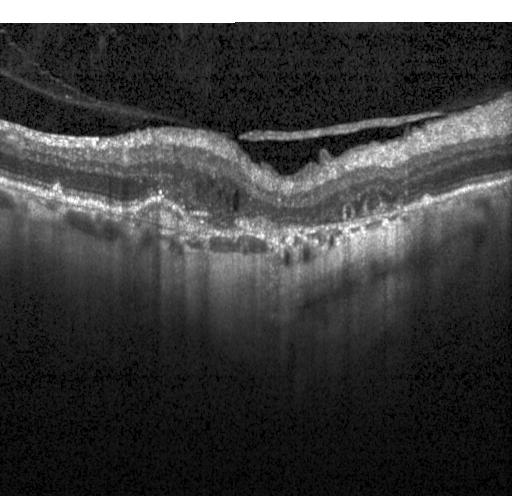 Macular OCT: a choroidal neovascular membrane.